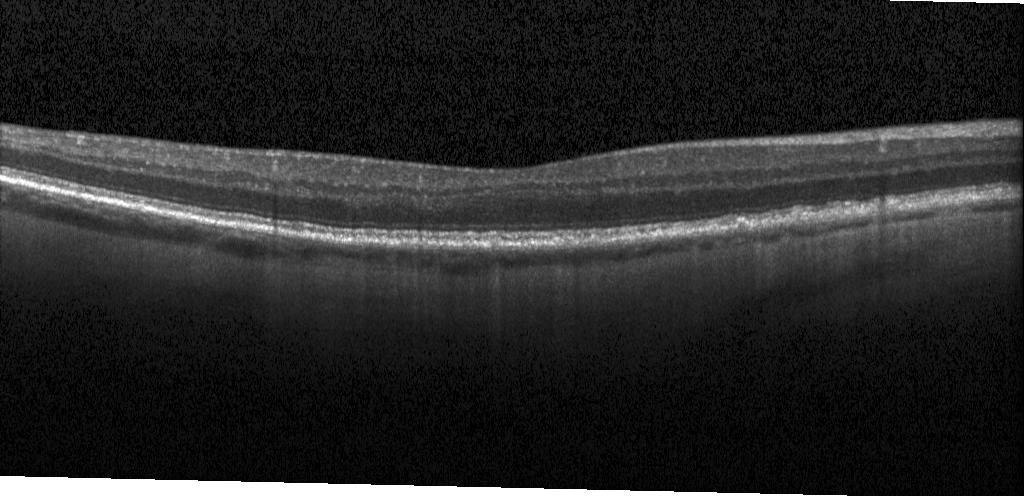

OCT B-scan, horizontal scan through the fovea, spectral-domain OCT. Diagnosis: drusen.